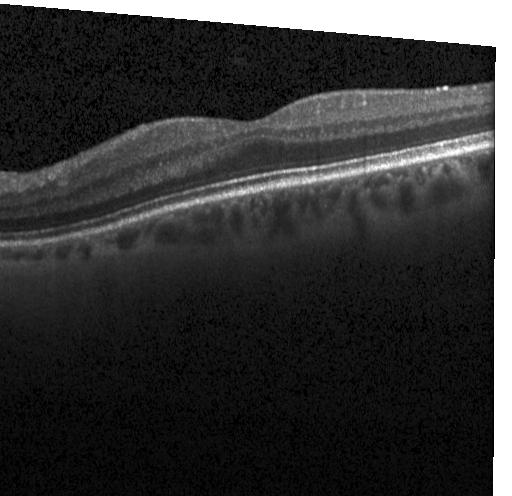
Optical coherence tomography B-scan.
Impression: no choroidal neovascularization, no diabetic macular edema, and no drusen.